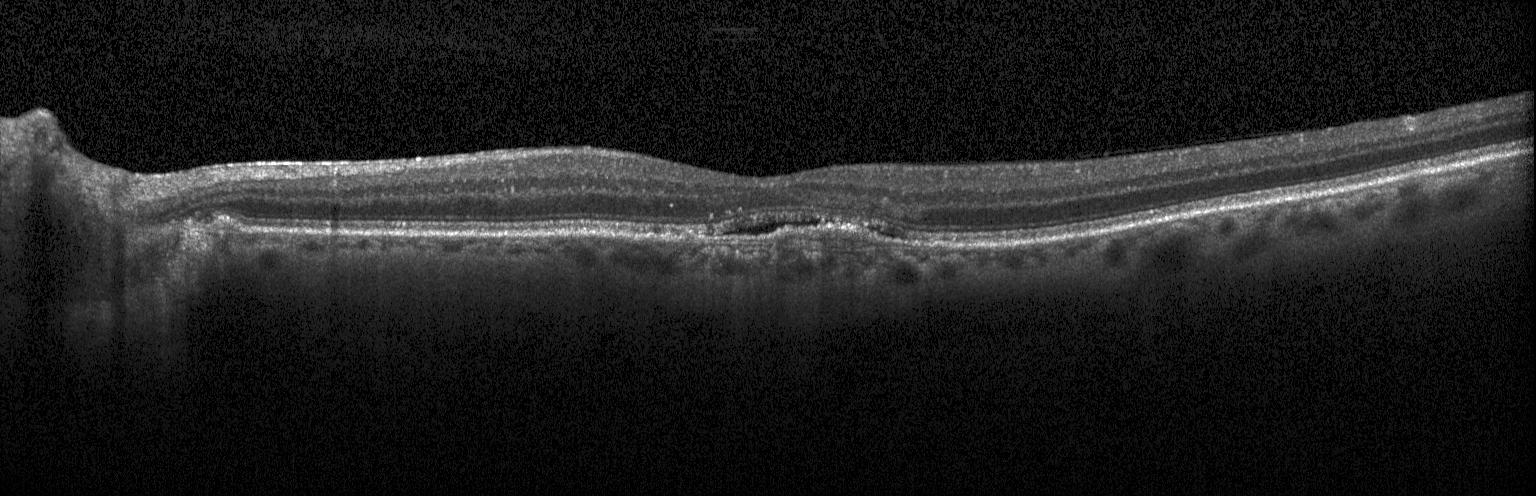
Fovea-centered; spectral-domain optical coherence tomography; Heidelberg Spectralis OCT system; retinal OCT B-scan.
This B-scan demonstrates CNV.